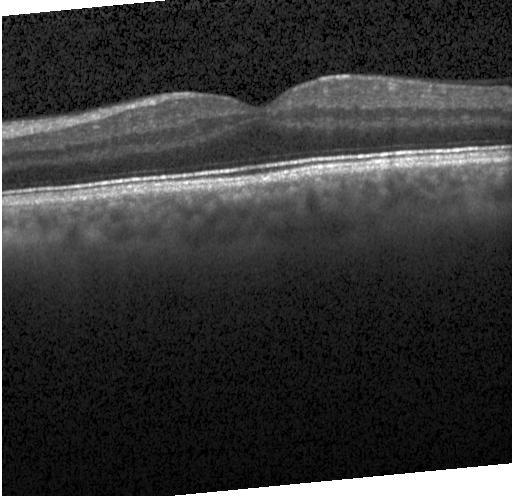
This B-scan demonstrates no choroidal neovascularization, diabetic macular edema, or drusen.